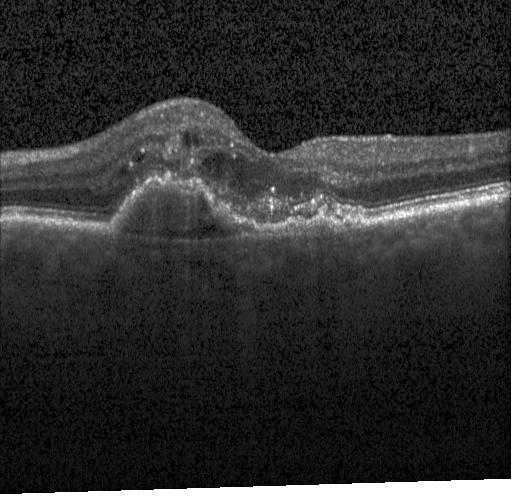 OCT line scan.
Impression: a choroidal neovascular membrane.